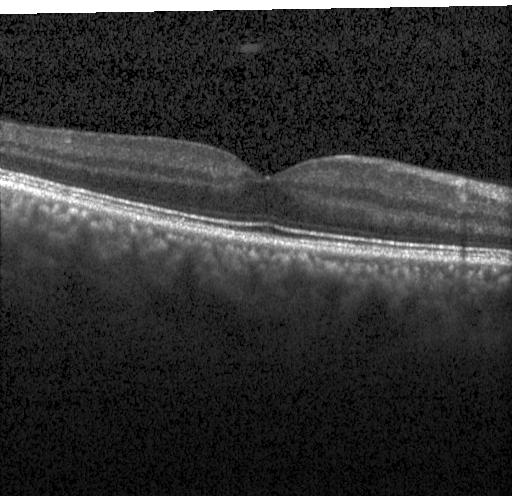

The scan shows neither choroidal neovascularization, diabetic macular edema, nor drusen.